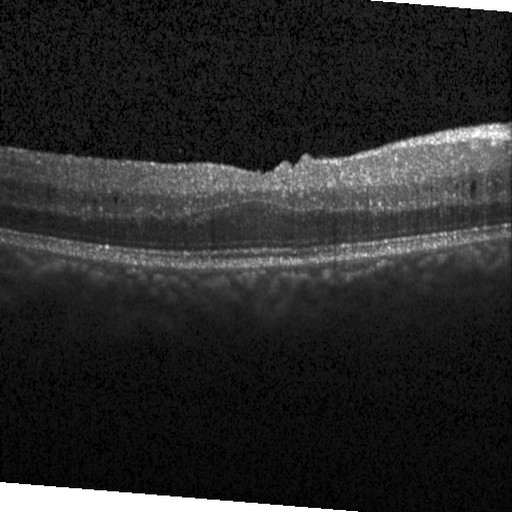

OCT B-scan; spectral-domain optical coherence tomography.
Impression: diabetic macular edema.